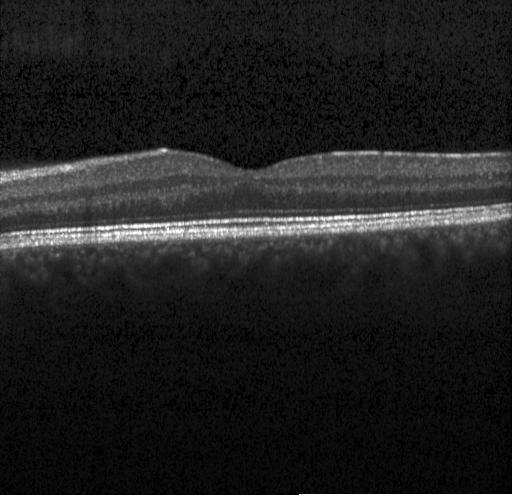

Heidelberg Spectralis · optical coherence tomography scan · centered on the fovea · spectral-domain optical coherence tomography — Finding: no choroidal neovascularization, no diabetic macular edema, and no drusen.